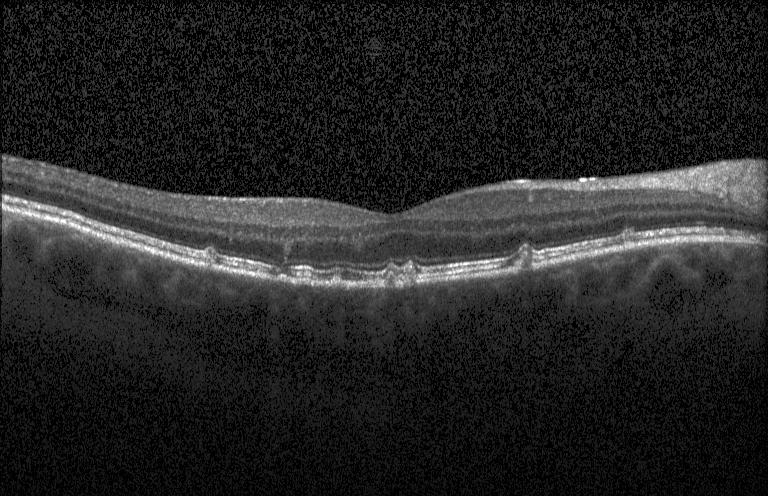

Optical coherence tomography B-scan, fovea-centered
This B-scan demonstrates multiple drusen.